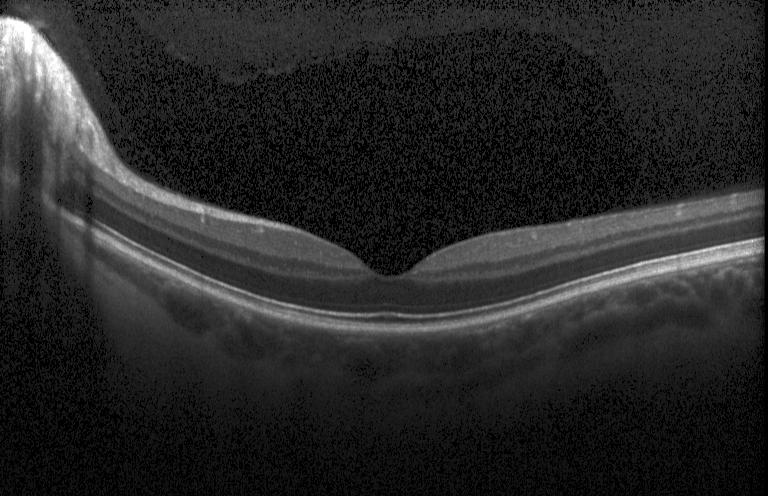 Diagnosis: no evidence of CNV, DME, or drusen.